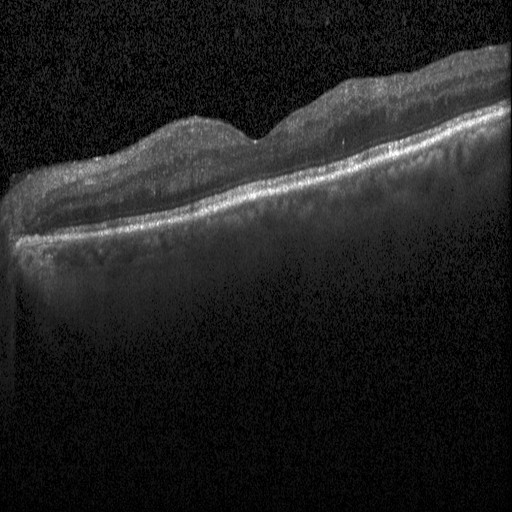 Finding: diabetic macular edema (DME).